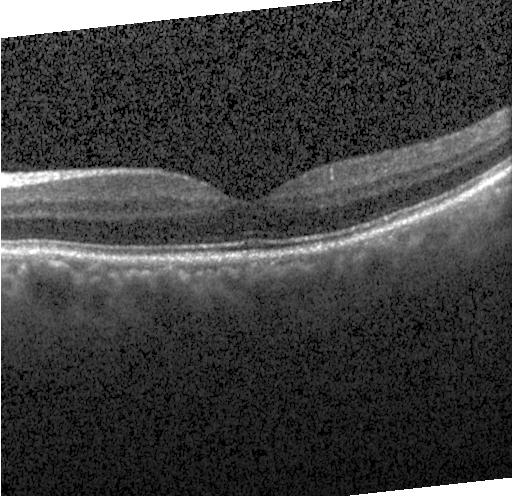 Macular OCT: no evidence of choroidal neovascularization, diabetic macular edema, or drusen.